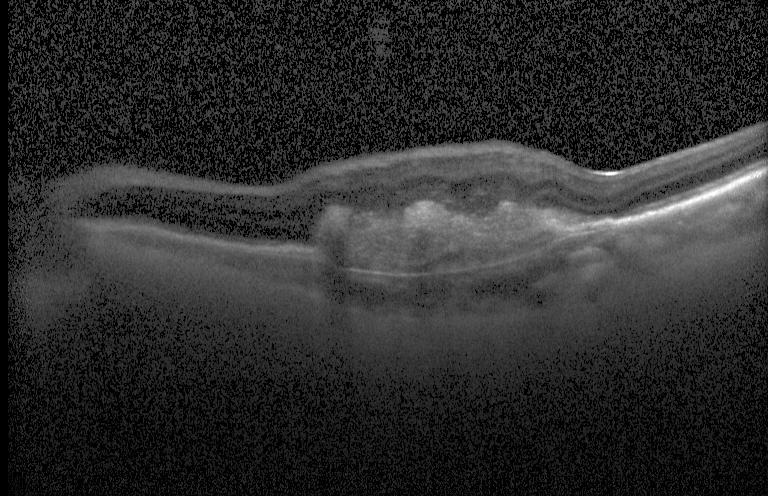
Impression: a choroidal neovascular membrane.